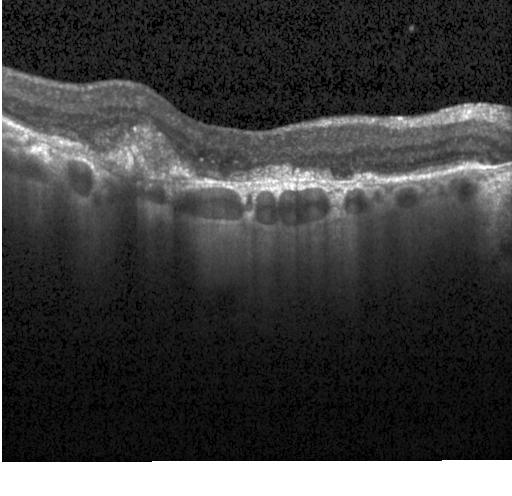
Instrument: Heidelberg Spectralis. Spectral-domain OCT. Retinal OCT B-scan. Horizontal scan through the fovea — Finding: choroidal neovascularization.